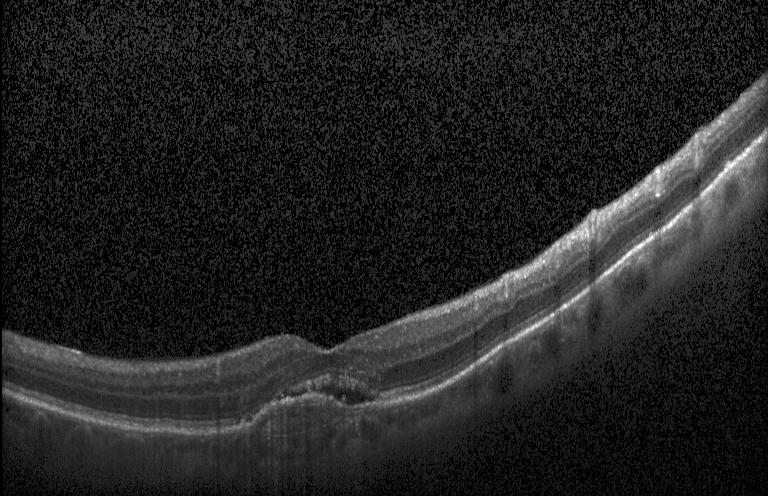

Retinal OCT cross-section. Macular OCT: a choroidal neovascular membrane.